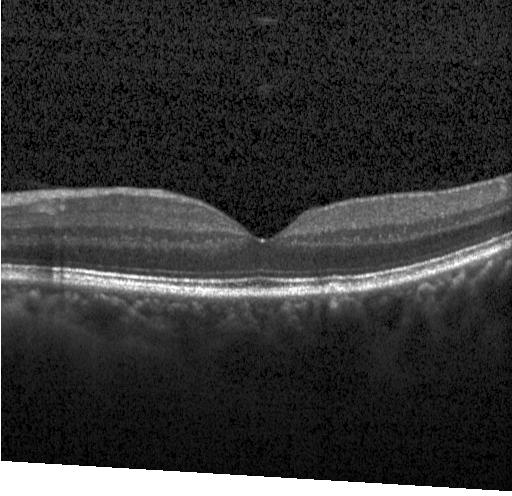
OCT B-scan, fovea-centered
This B-scan demonstrates no evidence of CNV, DME, or drusen.